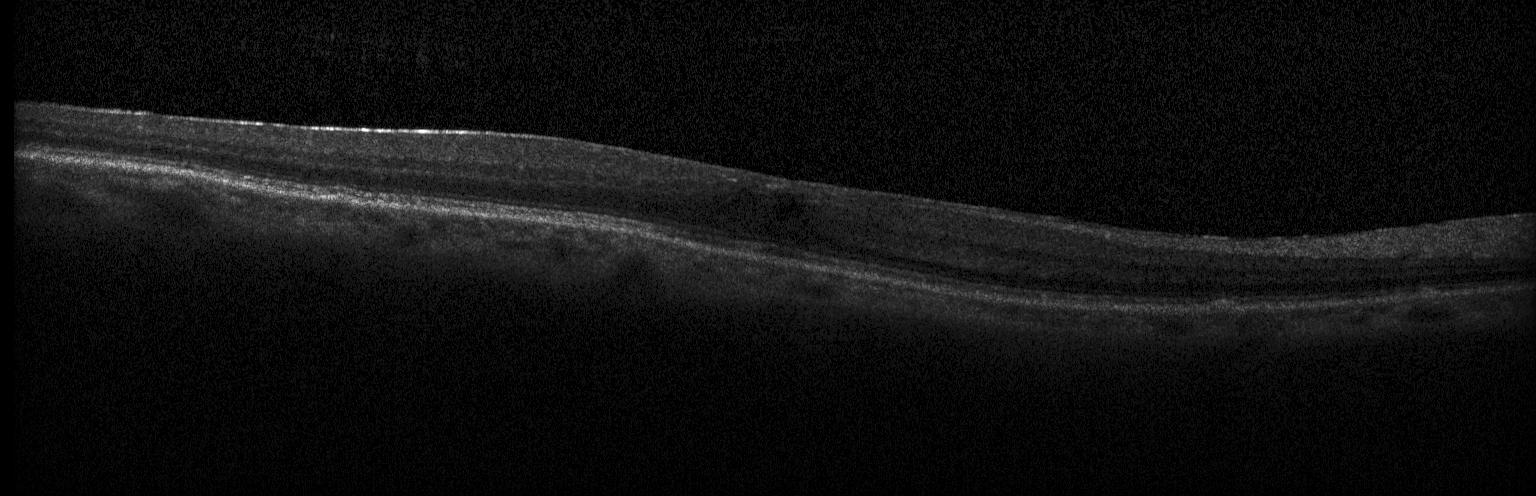
Retinal OCT cross-section showing diabetic macular edema.